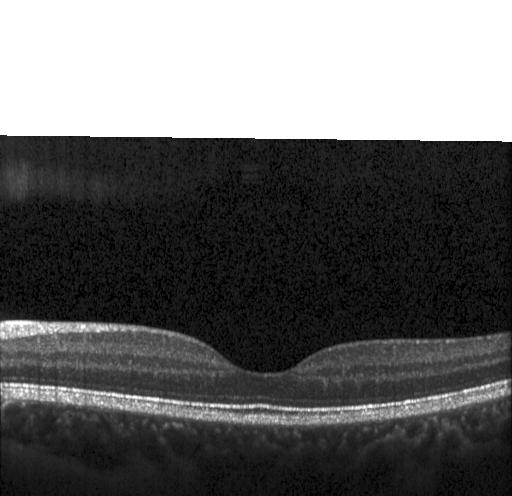 Heidelberg Spectralis OCT system; spectral-domain OCT; optical coherence tomography B-scan; macular scan
Assessment: no evidence of choroidal neovascularization, diabetic macular edema, or drusen.